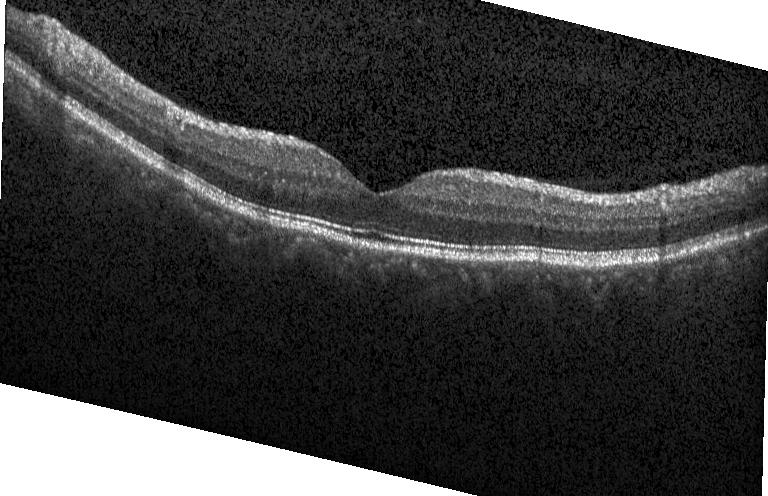
Impression: no CNV, no DME, and no drusen.